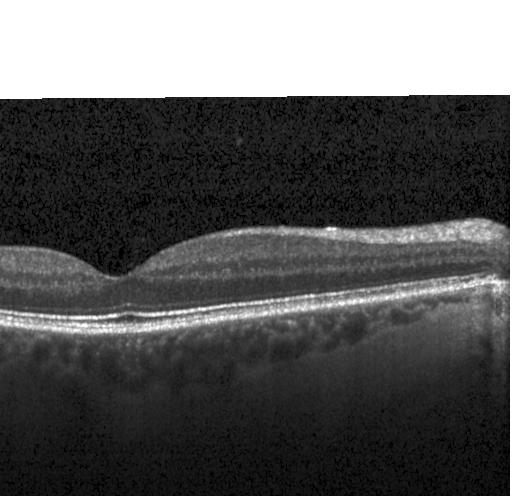
Optical coherence tomography B-scan. Impression: no choroidal neovascularization, no diabetic macular edema, and no drusen.